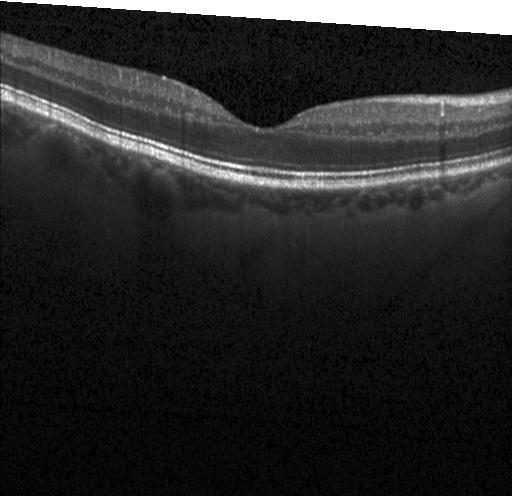
Optical coherence tomography B-scan
The scan shows no choroidal neovascularization, no diabetic macular edema, and no drusen.